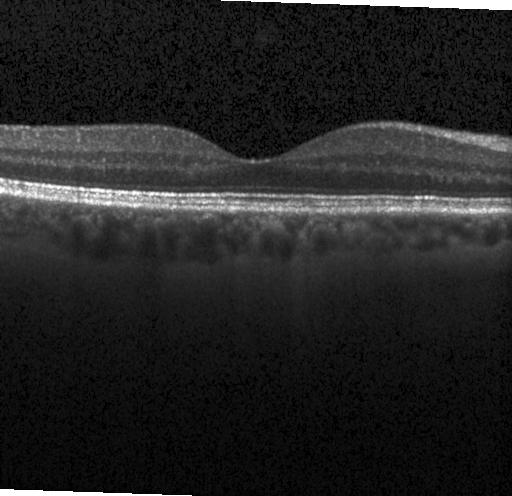
Macular OCT: neither choroidal neovascularization, diabetic macular edema, nor drusen.